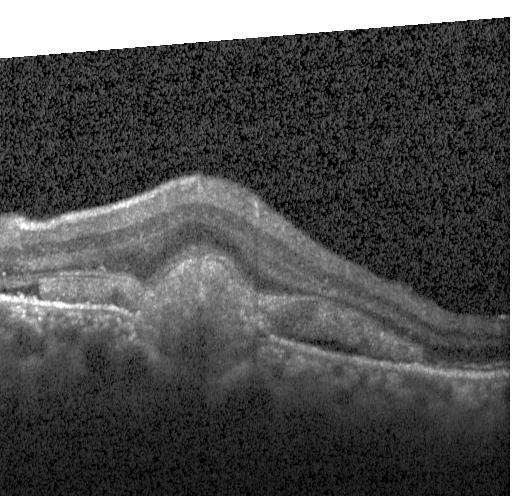 Retinal OCT B-scan.
Diagnosis: choroidal neovascularization.